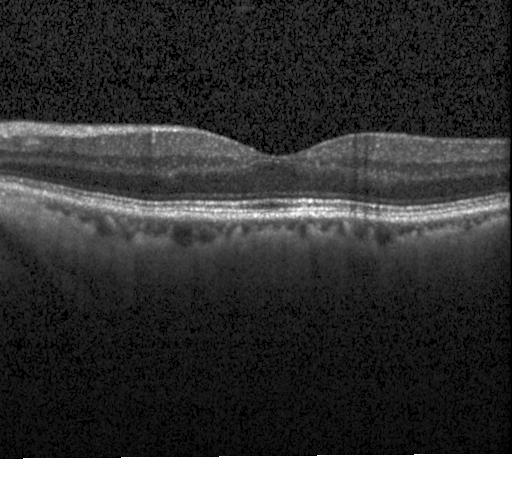

Macular OCT demonstrating no evidence of CNV, DME, or drusen.